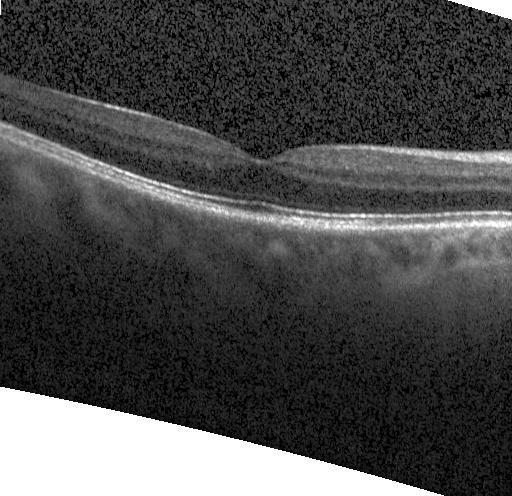
Impression: no evidence of choroidal neovascularization, diabetic macular edema, or drusen.